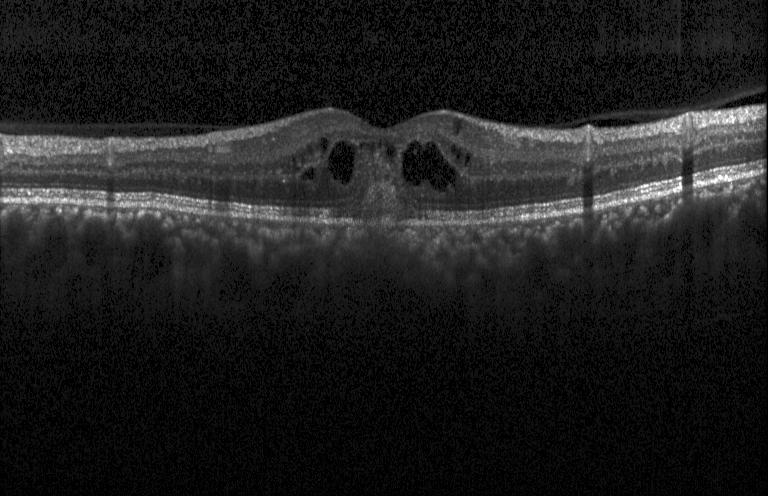 Optical coherence tomography scan; spectral-domain optical coherence tomography; macular scan. Macular OCT: a choroidal neovascular membrane.